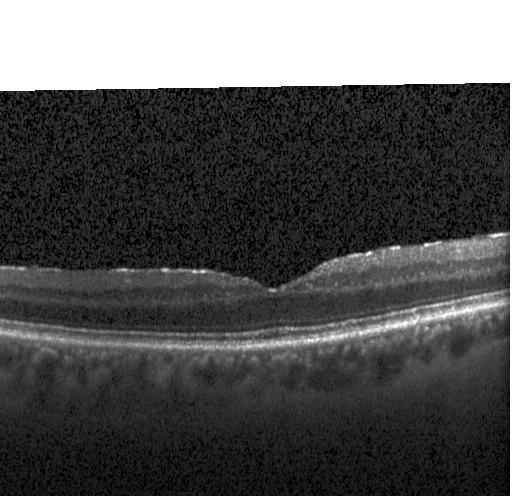

SD-OCT; Heidelberg Spectralis; retinal OCT B-scan. Assessment: no CNV, no DME, and no drusen.